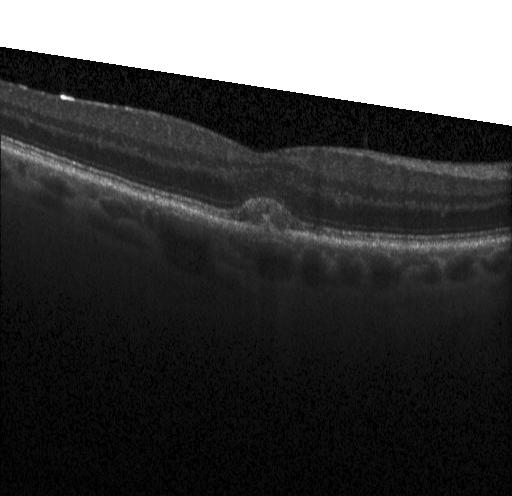
SD-OCT; optical coherence tomography B-scan; Heidelberg Spectralis. Macular OCT: CNV.